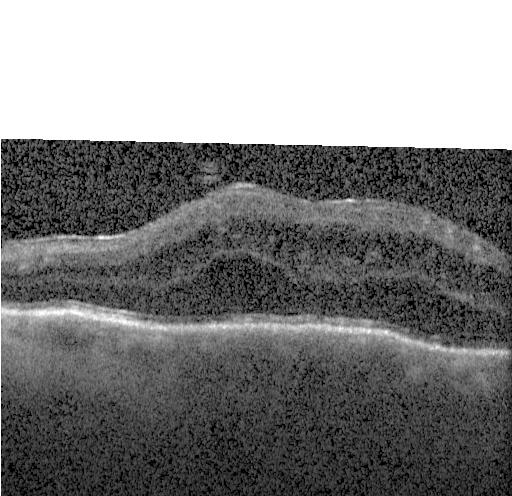 SD-OCT; Heidelberg Spectralis OCT system; retinal OCT cross-section — This B-scan demonstrates diabetic macular edema (DME).